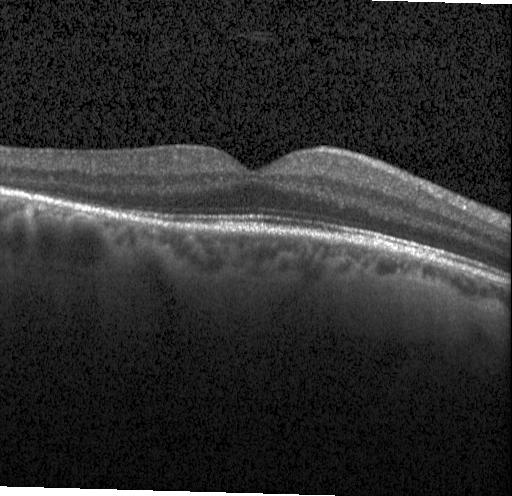 Spectral-domain OCT; centered on the fovea; optical coherence tomography B-scan; Heidelberg Spectralis.
Impression: neither CNV, DME, nor drusen.